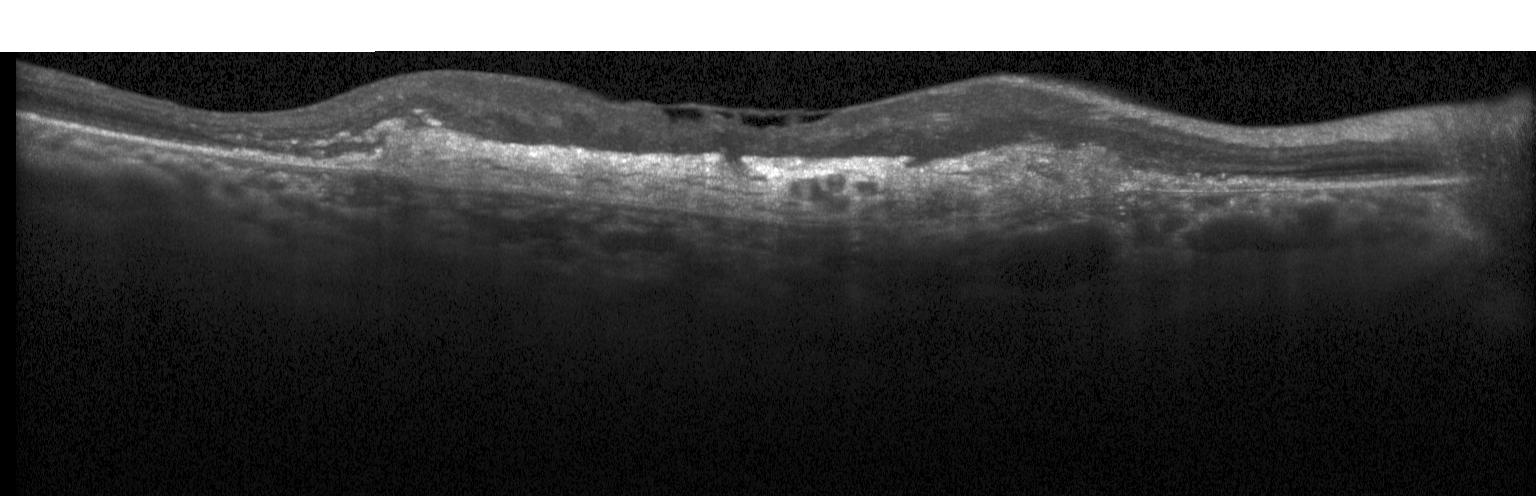
Spectral-domain OCT B-scan: a choroidal neovascular membrane.